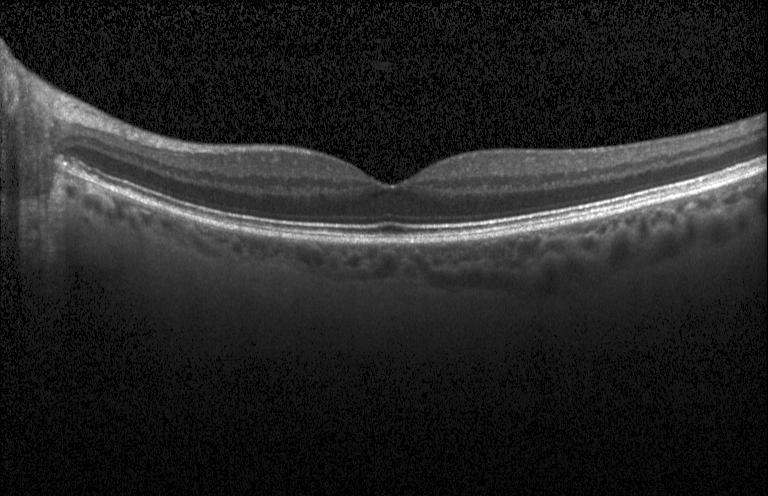 Macular scan; Heidelberg Spectralis; retinal OCT cross-section — Impression: no CNV, no DME, and no drusen.